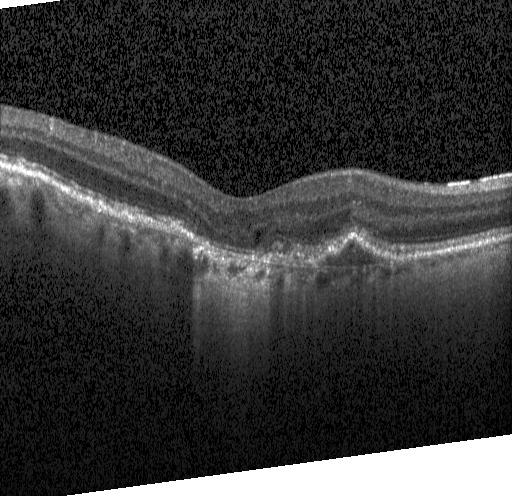 Optical coherence tomography B-scan — Impression: choroidal neovascularization (CNV).